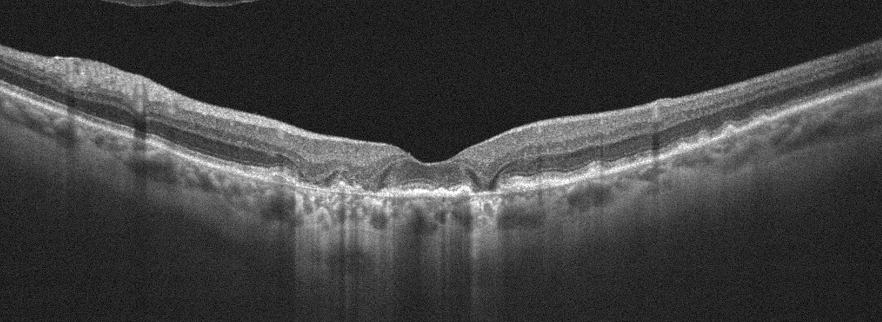

Instrument: Optovue Avanti RTVue XR · OCT B-scan · left eye · through the macula — Macular OCT: AMD.